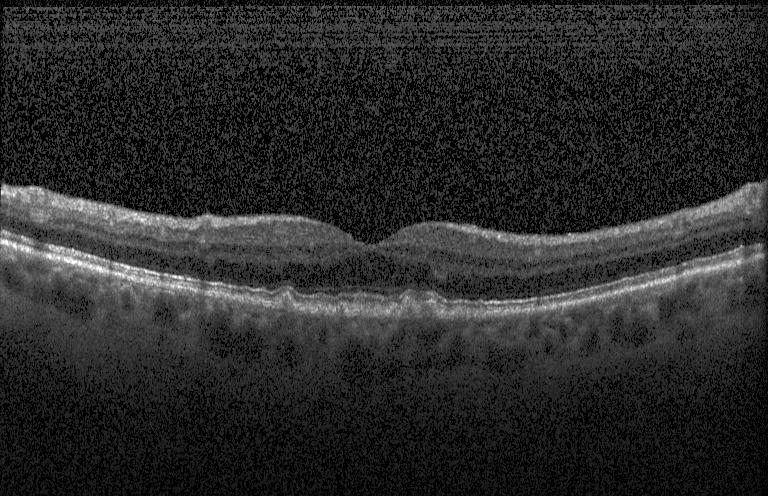

Spectral-domain OCT. Heidelberg Spectralis OCT system. Through the macula. Retinal OCT B-scan — Assessment: sub-RPE drusenoid deposits.